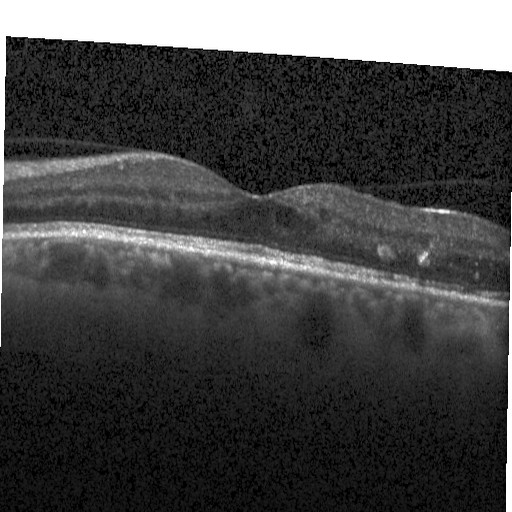 Retinal OCT B-scan; Heidelberg Spectralis; spectral-domain OCT.
DME.